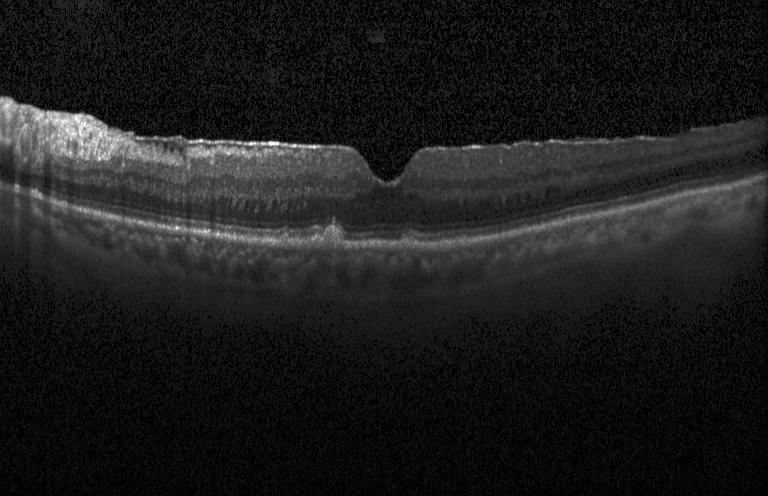
Retinal OCT cross-section · fovea-centered · Heidelberg Spectralis
The scan shows drusen.